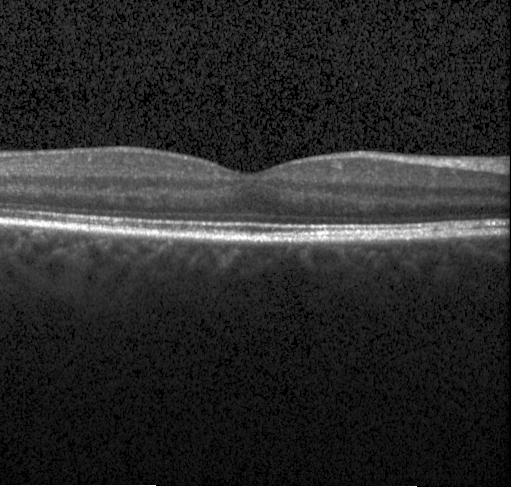

Finding: no choroidal neovascularization, no diabetic macular edema, and no drusen.